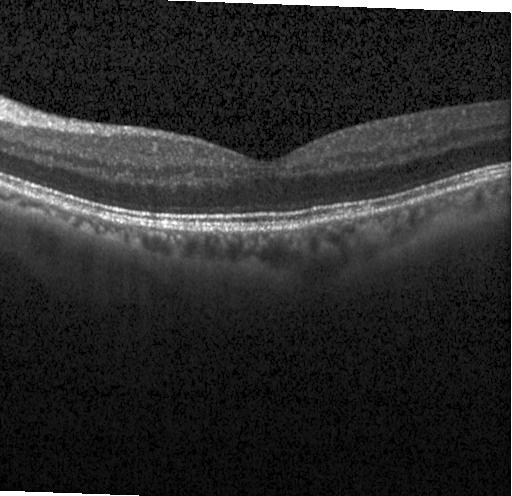 OCT line scan. Spectral-domain OCT. Instrument: Heidelberg Spectralis. Finding: no CNV, DME, or drusen.